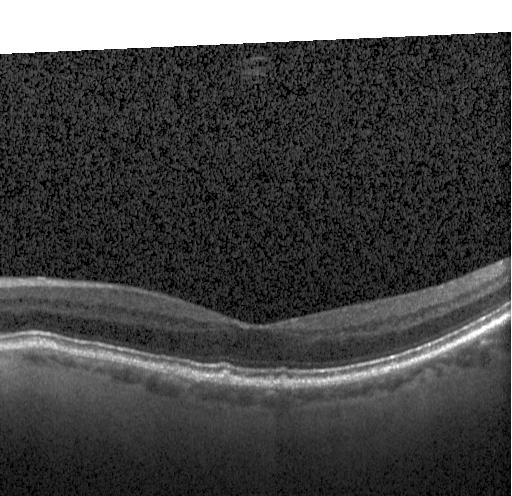
Spectral-domain OCT B-scan: sub-RPE drusenoid deposits.